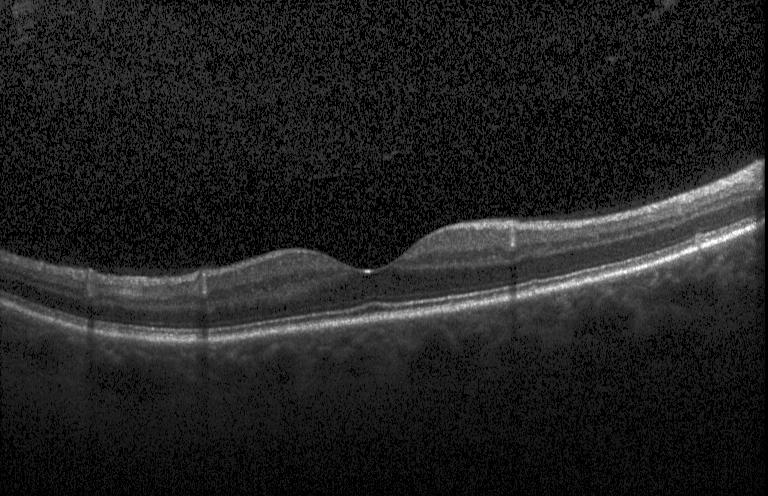

Acquired on a Heidelberg Spectralis; horizontal scan through the fovea; optical coherence tomography scan.
The scan shows sub-RPE drusenoid deposits.